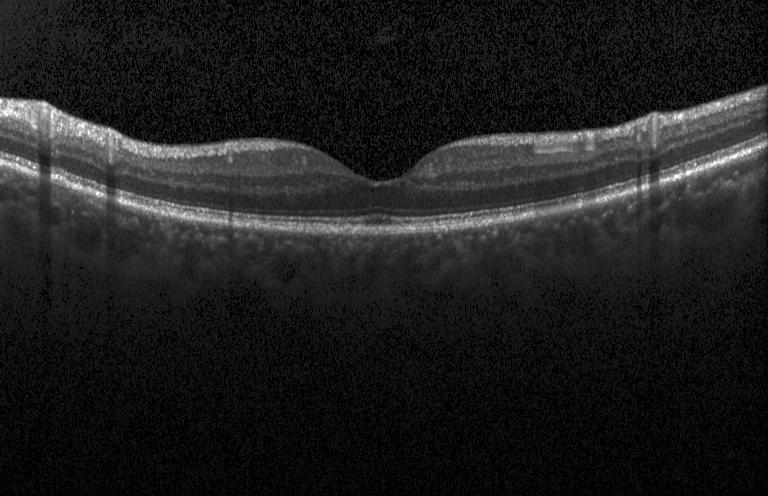

No CNV, no DME, and no drusen.